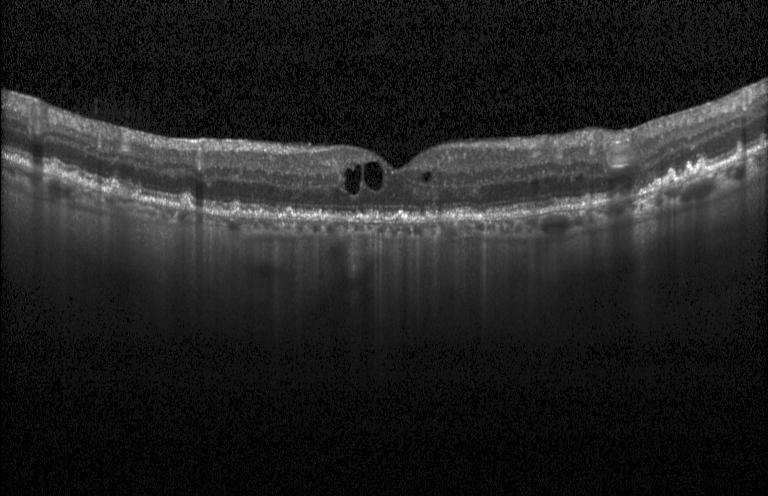
Dx: a choroidal neovascular membrane.